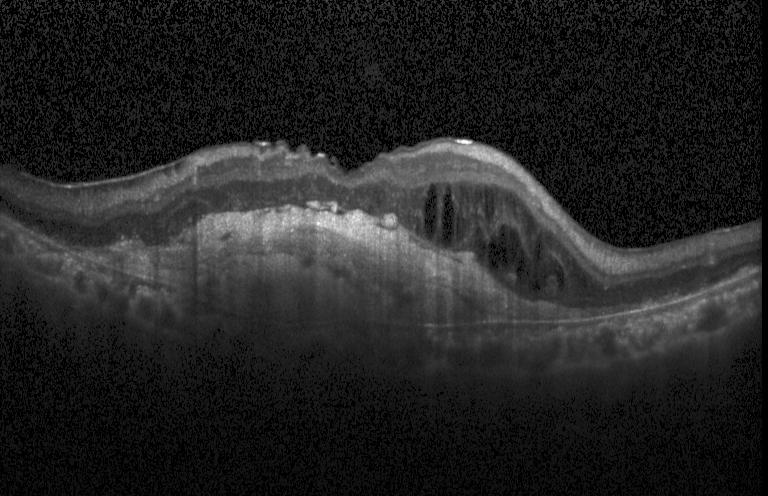
OCT line scan. Spectral-domain optical coherence tomography. Fovea-centered. Heidelberg Spectralis OCT system — Dx: choroidal neovascularization.